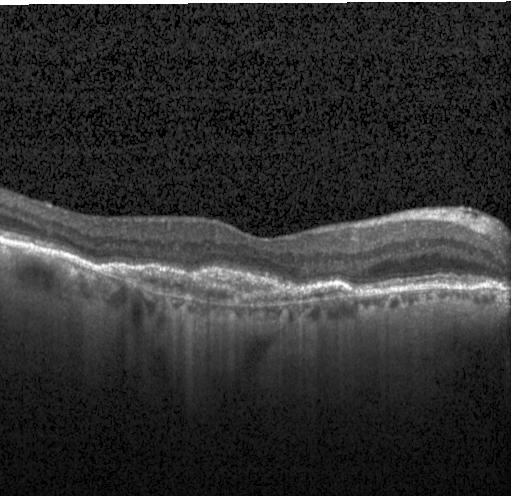
OCT line scan. Spectral-domain OCT. Macular scan.
A choroidal neovascular membrane.